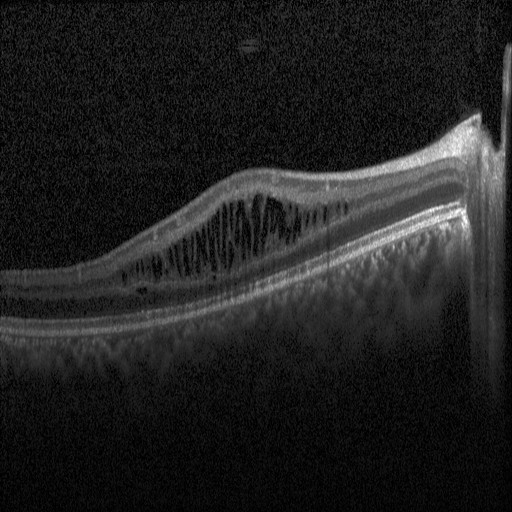 Retinal OCT cross-section · through the macula — Assessment: diabetic macular edema.